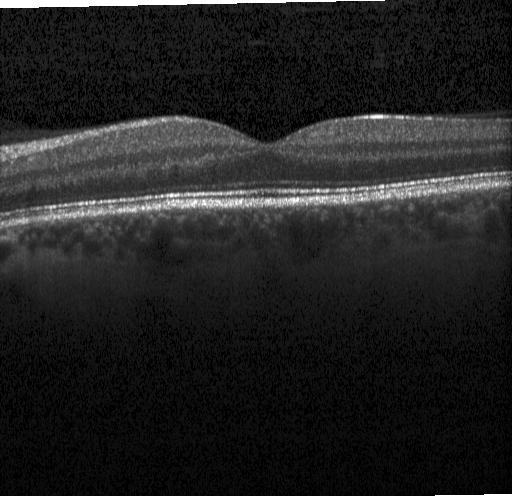 Spectral-domain optical coherence tomography; acquired on a Heidelberg Spectralis; optical coherence tomography B-scan.
Finding: no CNV, DME, or drusen.